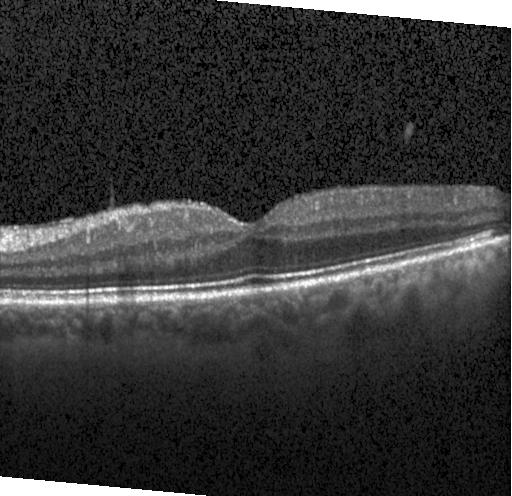

This B-scan demonstrates no choroidal neovascularization, diabetic macular edema, or drusen.